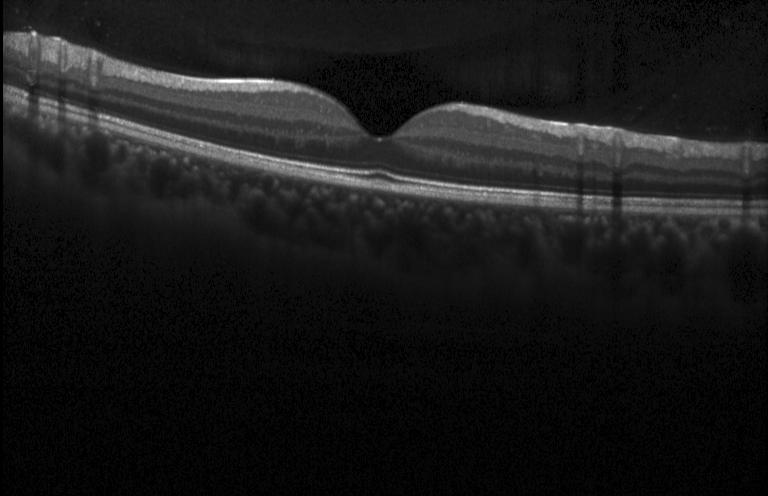

Dx: no evidence of choroidal neovascularization, diabetic macular edema, or drusen.